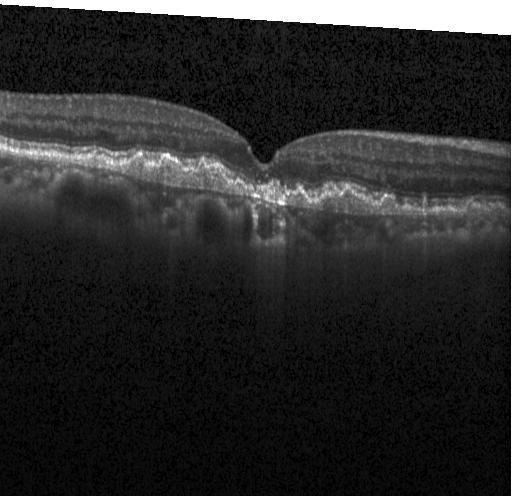

Retinal OCT B-scan; SD-OCT; fovea-centered; Heidelberg Spectralis OCT system.
Finding: a choroidal neovascular membrane.